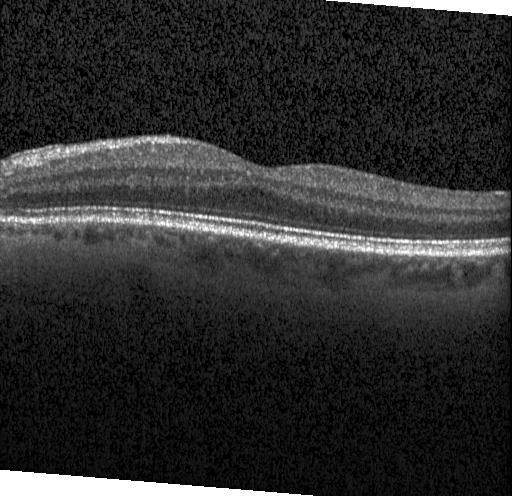 Spectral-domain OCT B-scan: no CNV, DME, or drusen.